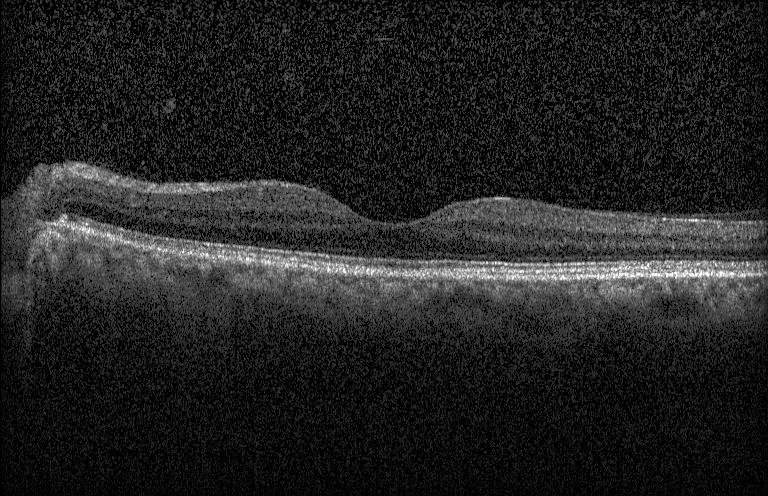
OCT B-scan. Spectral-domain optical coherence tomography. Heidelberg Spectralis OCT system. Macular scan — Finding: neither CNV, DME, nor drusen.